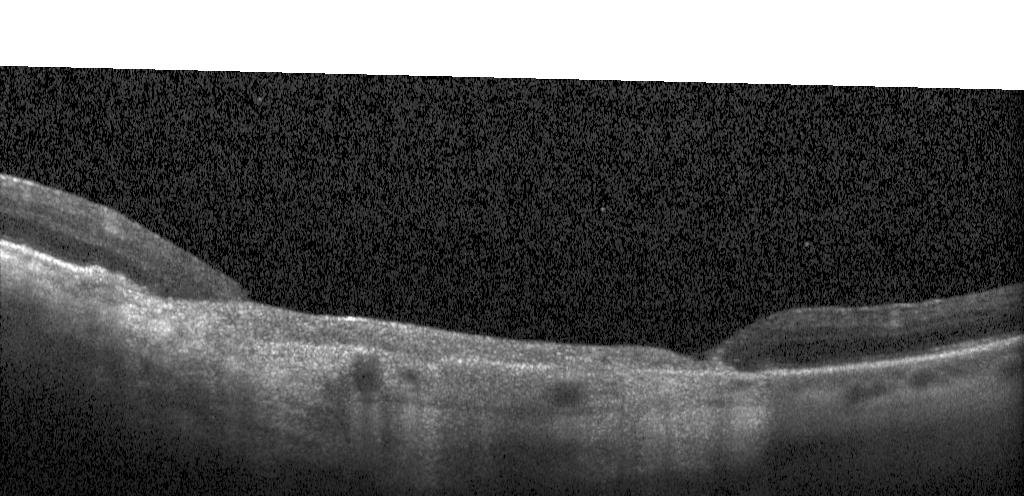
Spectral-domain optical coherence tomography · through the macula · retinal OCT cross-section · instrument: Heidelberg Spectralis.
Impression: CNV.